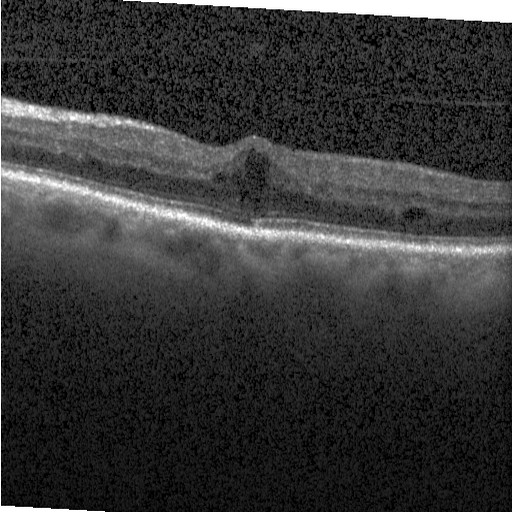 Impression: DME.